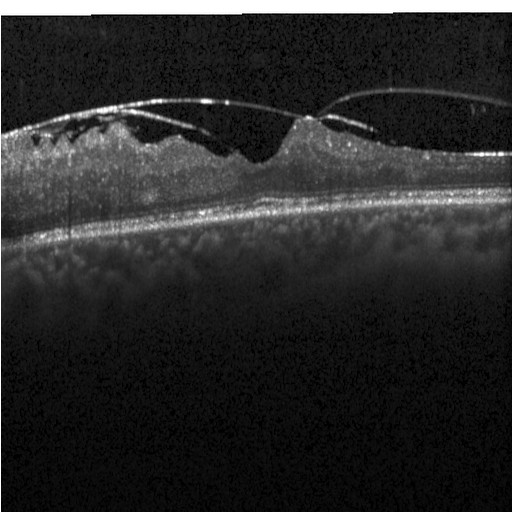

Finding: diabetic macular edema (DME).